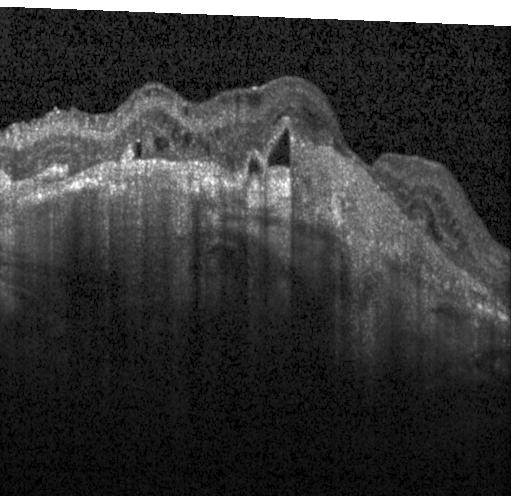 Optical coherence tomography scan
This B-scan demonstrates a choroidal neovascular membrane.